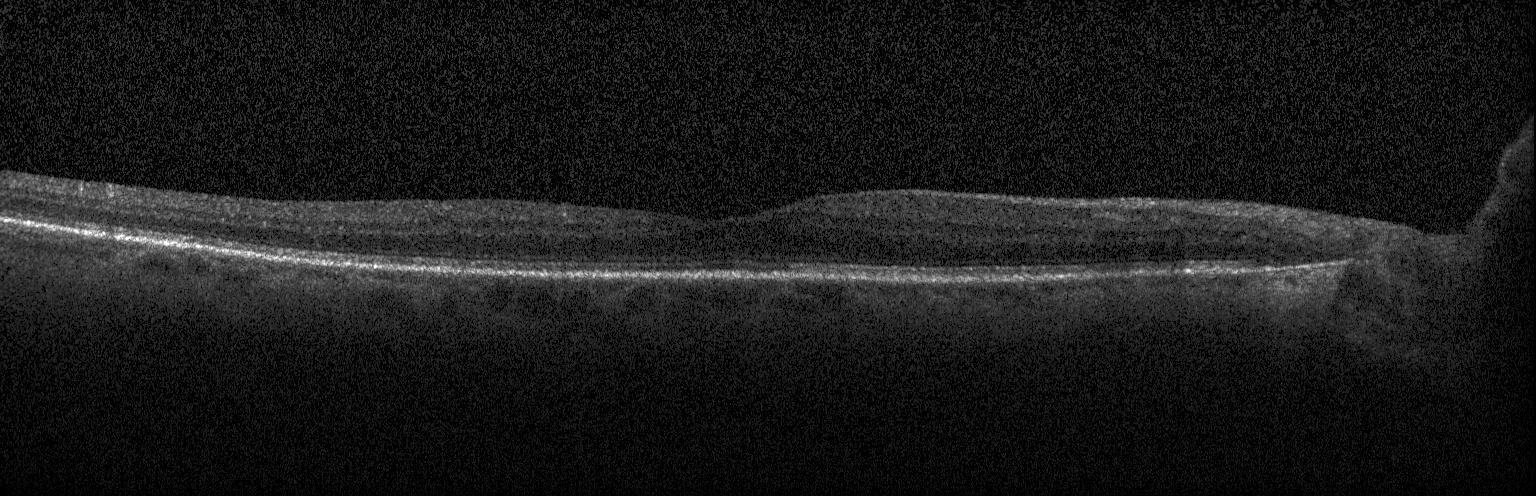 OCT line scan. Heidelberg Spectralis OCT system. Horizontal scan through the fovea. OCT finding: no choroidal neovascularization, no diabetic macular edema, and no drusen.